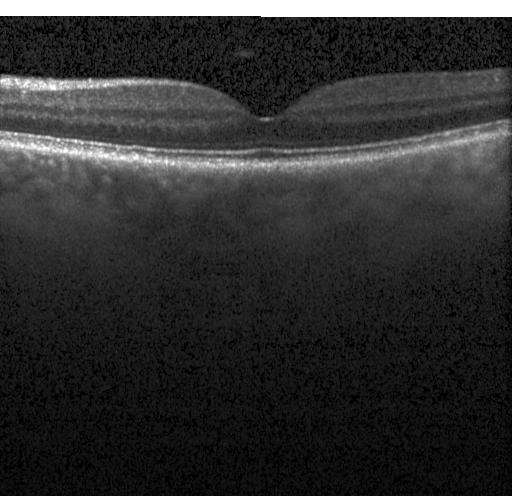

OCT line scan
Diagnosis: no choroidal neovascularization, no diabetic macular edema, and no drusen.